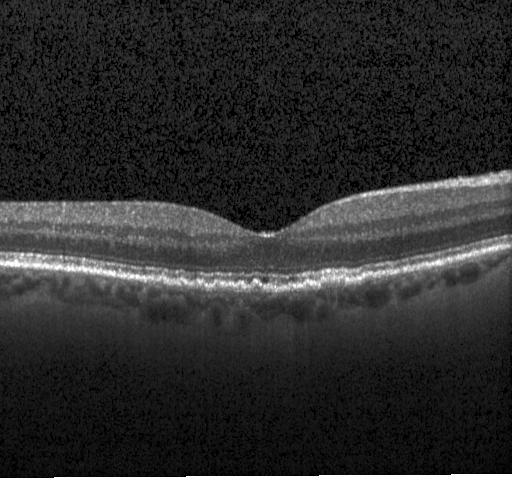 Horizontal scan through the fovea. Spectral-domain optical coherence tomography. Optical coherence tomography scan. Dx: multiple drusen.